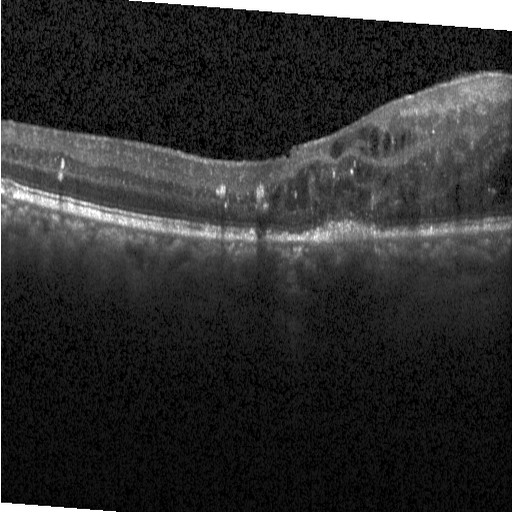 Finding: diabetic macular edema (DME).